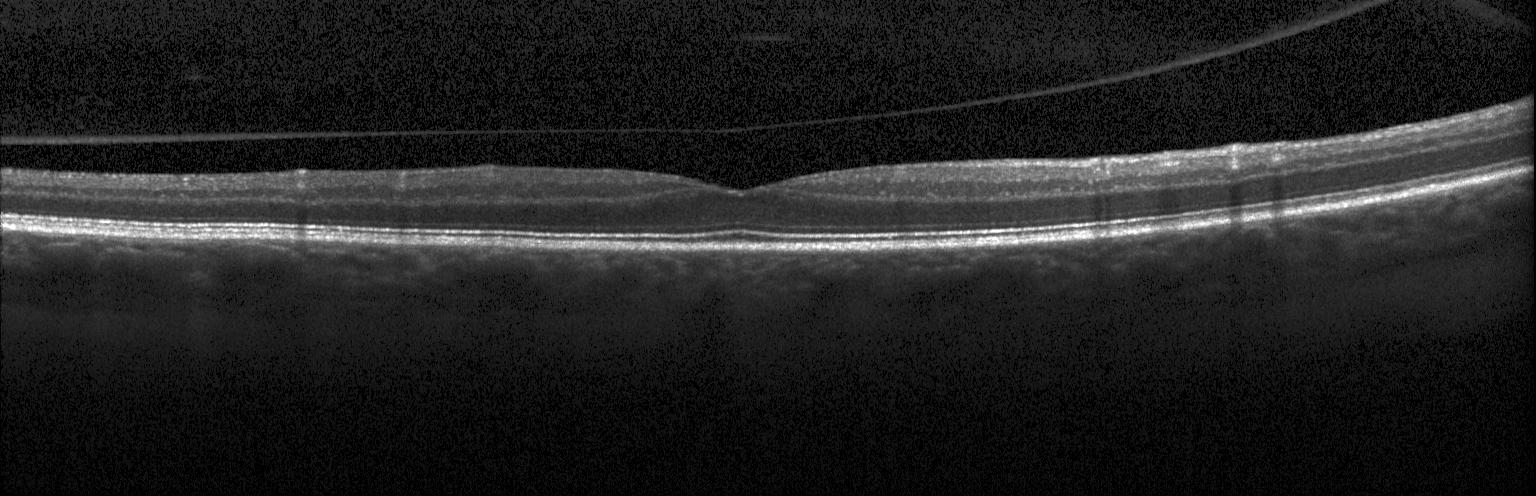 Impression: no choroidal neovascularization, no diabetic macular edema, and no drusen.